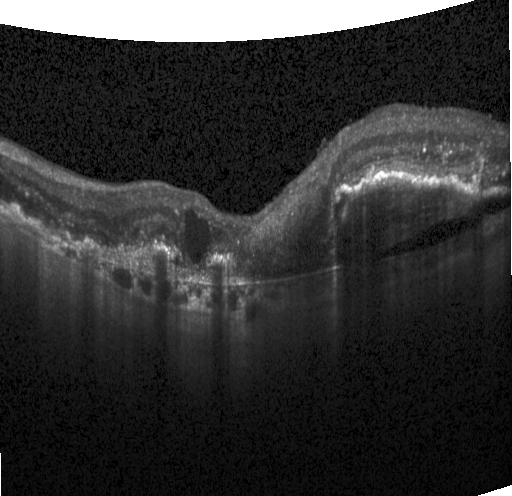 Instrument: Heidelberg Spectralis · spectral-domain optical coherence tomography · OCT line scan · horizontal scan through the fovea — Assessment: CNV.